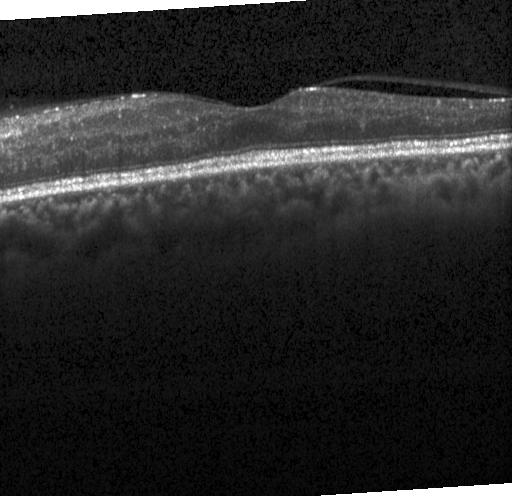 Centered on the fovea; Heidelberg Spectralis OCT system; spectral-domain OCT; optical coherence tomography scan.
Finding: diabetic macular edema.